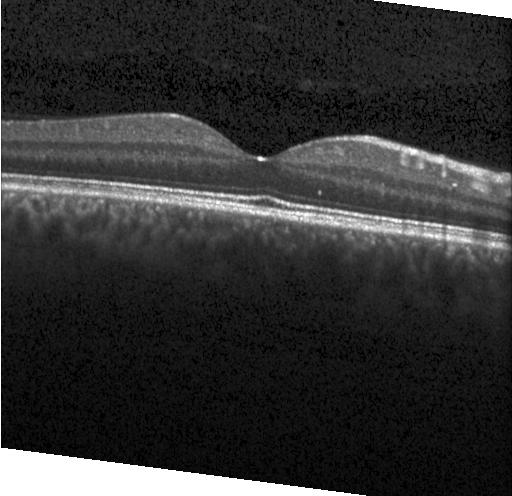
Optical coherence tomography scan.
Impression: no CNV, no DME, and no drusen.